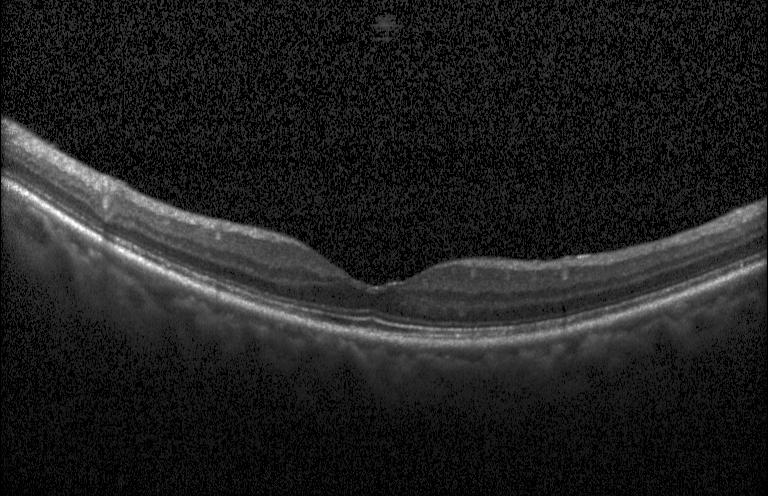
Finding: no choroidal neovascularization, no diabetic macular edema, and no drusen.